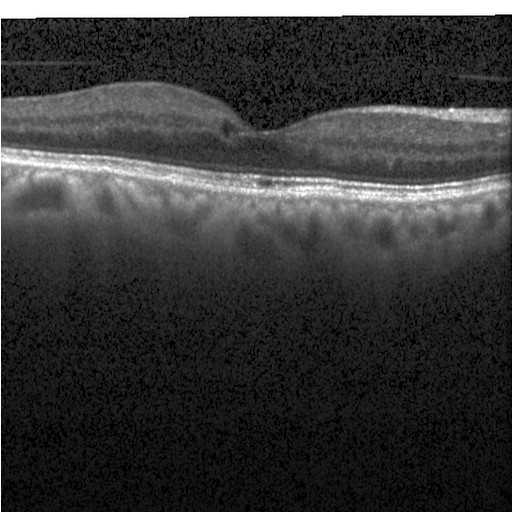
Centered on the fovea. Acquired on a Heidelberg Spectralis. Spectral-domain optical coherence tomography. Retinal OCT cross-section. Diagnosis: diabetic macular edema.